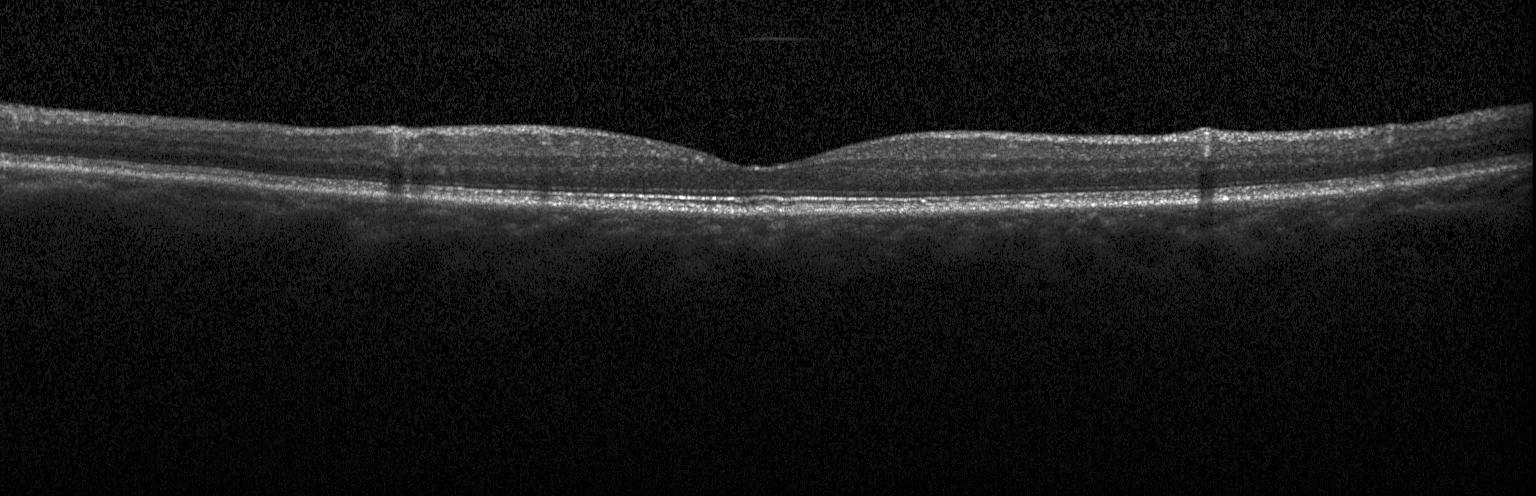 Spectral-domain optical coherence tomography, optical coherence tomography B-scan. Macular OCT: no CNV, DME, or drusen.